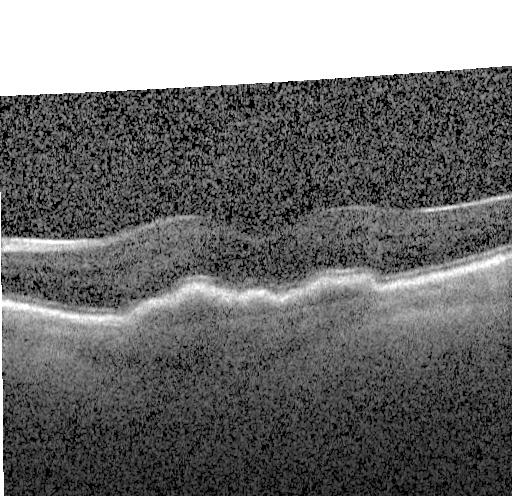
Diagnosis: CNV.